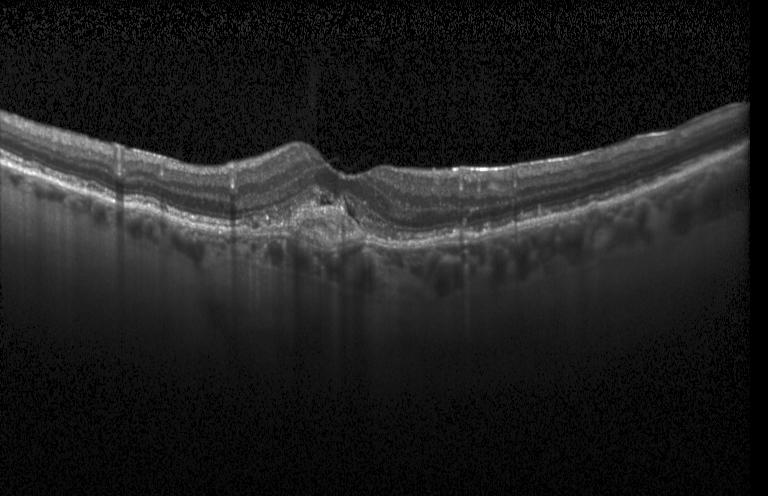
Centered on the fovea · retinal OCT B-scan · spectral-domain OCT. Macular OCT: a choroidal neovascular membrane.